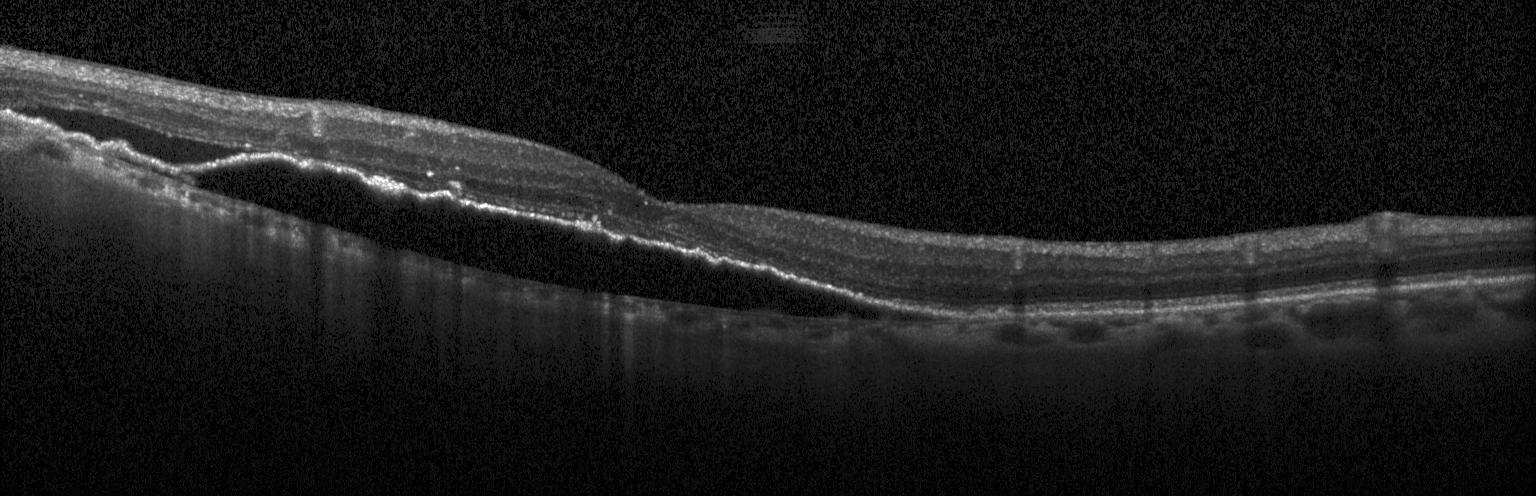

Spectral-domain OCT, optical coherence tomography B-scan — Impression: choroidal neovascularization (CNV).